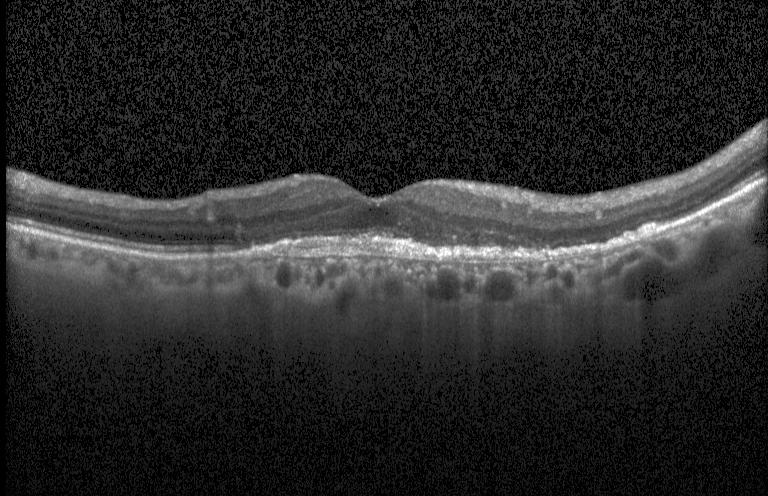
Fovea-centered. OCT line scan. Spectral-domain optical coherence tomography. Instrument: Heidelberg Spectralis.
This B-scan demonstrates choroidal neovascularization (CNV).